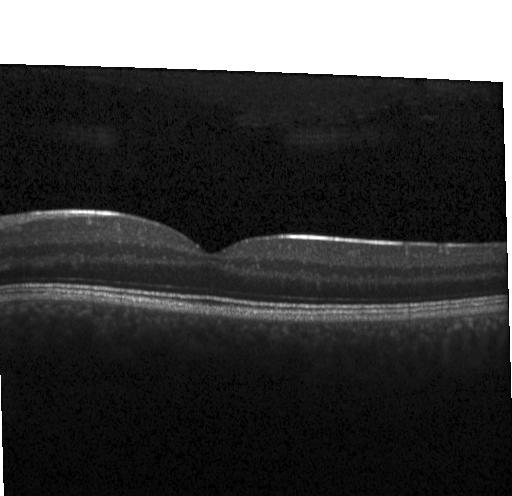
OCT finding: no evidence of CNV, DME, or drusen.